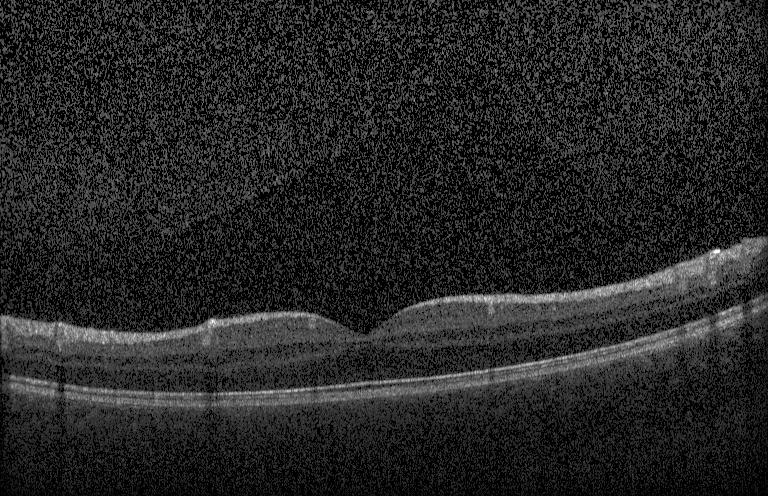 Macular OCT: no choroidal neovascularization, diabetic macular edema, or drusen.